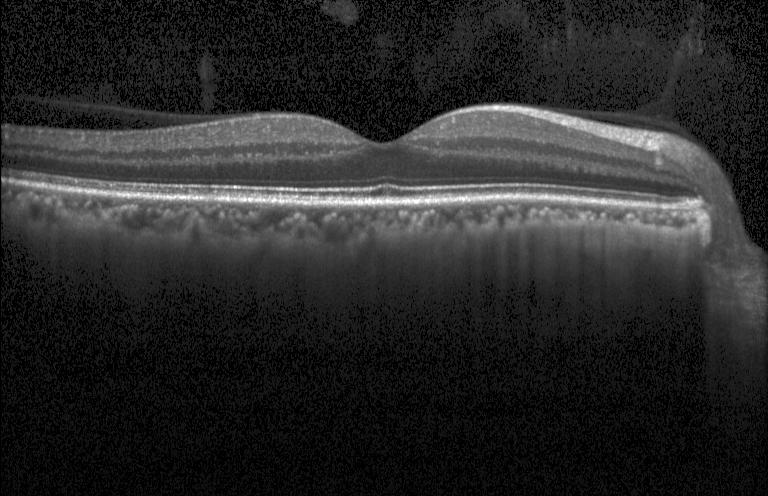

Spectral-domain optical coherence tomography; OCT B-scan; acquired on a Heidelberg Spectralis; macular scan
This B-scan demonstrates no choroidal neovascularization, no diabetic macular edema, and no drusen.